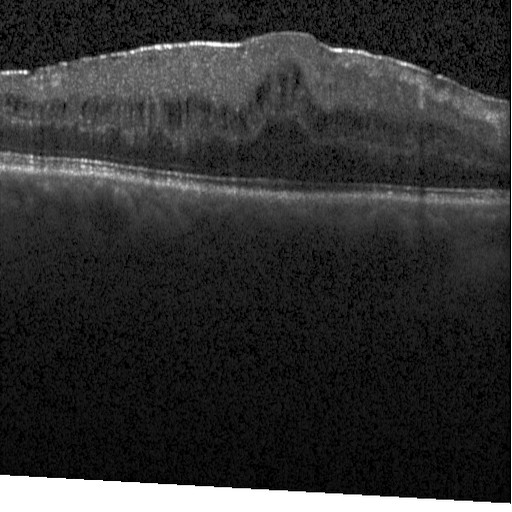

Impression: diabetic macular edema (DME).